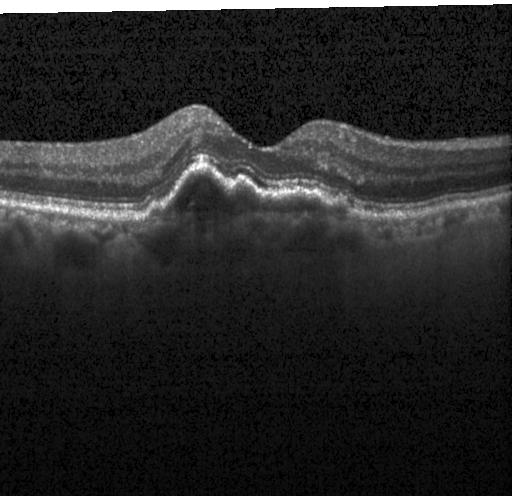 Finding: a choroidal neovascular membrane.